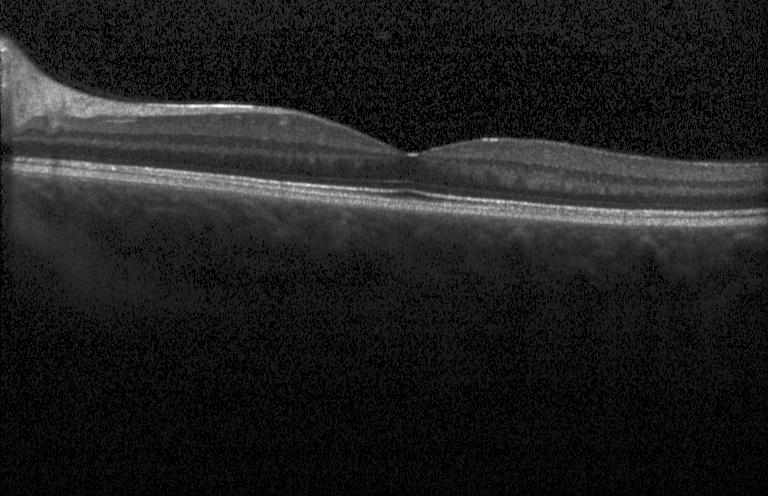

This B-scan demonstrates no choroidal neovascularization, no diabetic macular edema, and no drusen.